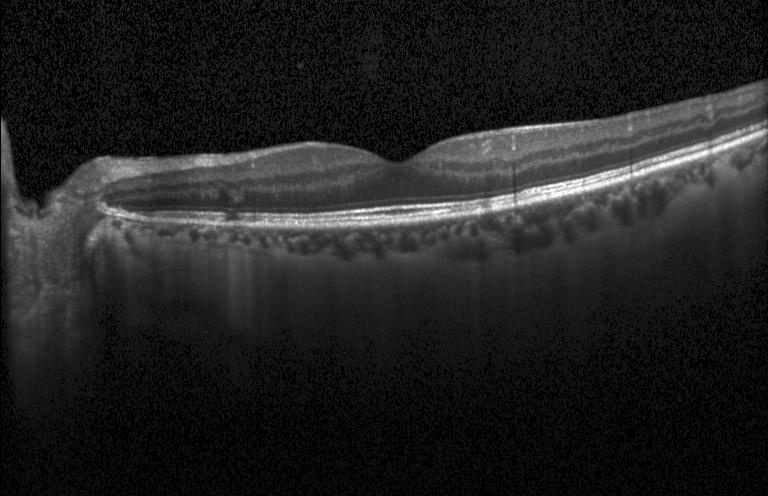 The scan shows no evidence of choroidal neovascularization, diabetic macular edema, or drusen.